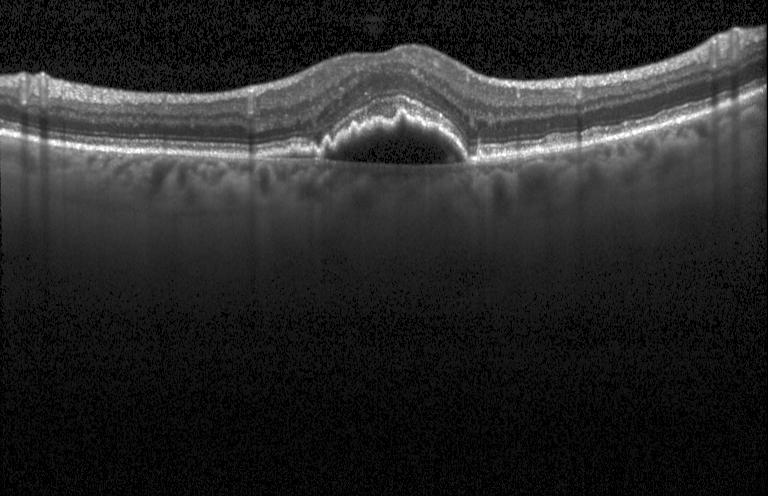

Acquired on a Heidelberg Spectralis, retinal OCT cross-section
The scan shows a choroidal neovascular membrane.